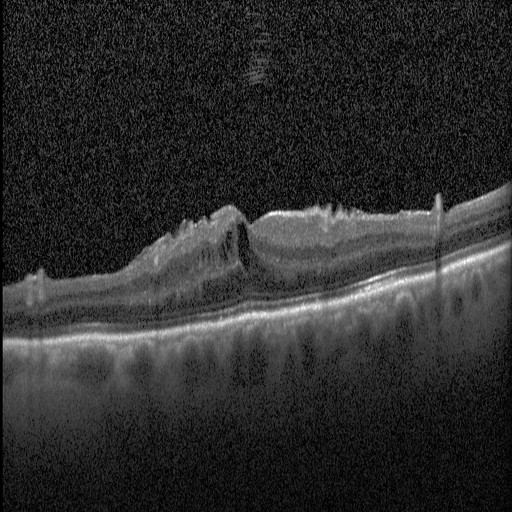 Instrument: Heidelberg Spectralis. Horizontal scan through the fovea. Spectral-domain optical coherence tomography. Optical coherence tomography B-scan.
Diagnosis: DME.